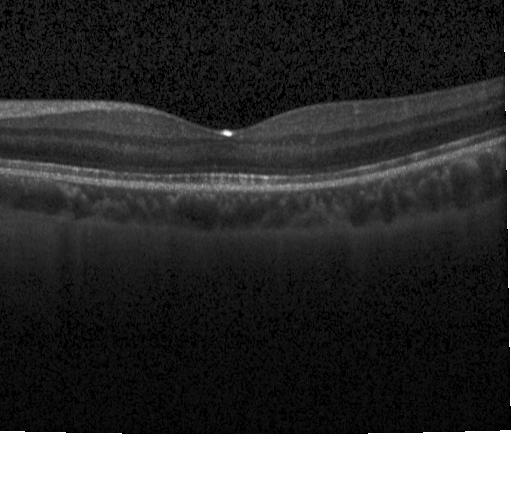
Neither choroidal neovascularization, diabetic macular edema, nor drusen.